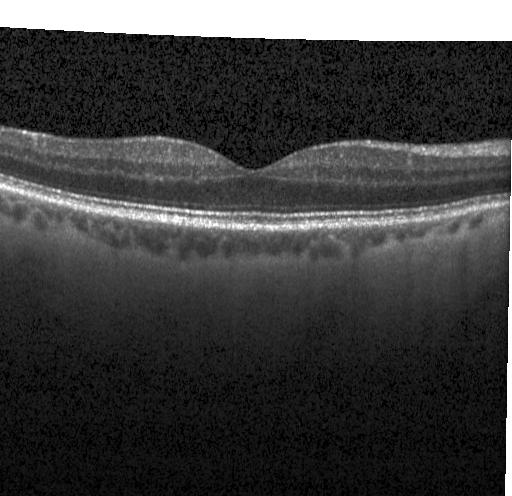 Spectral-domain optical coherence tomography. Heidelberg Spectralis. Macular scan. OCT line scan — Macular OCT: no choroidal neovascularization, no diabetic macular edema, and no drusen.